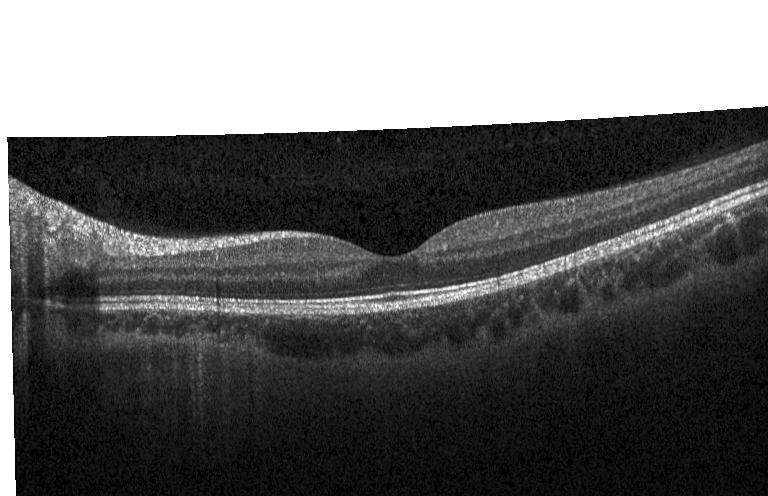
Through the macula · instrument: Heidelberg Spectralis · OCT B-scan.
Impression: no evidence of CNV, DME, or drusen.